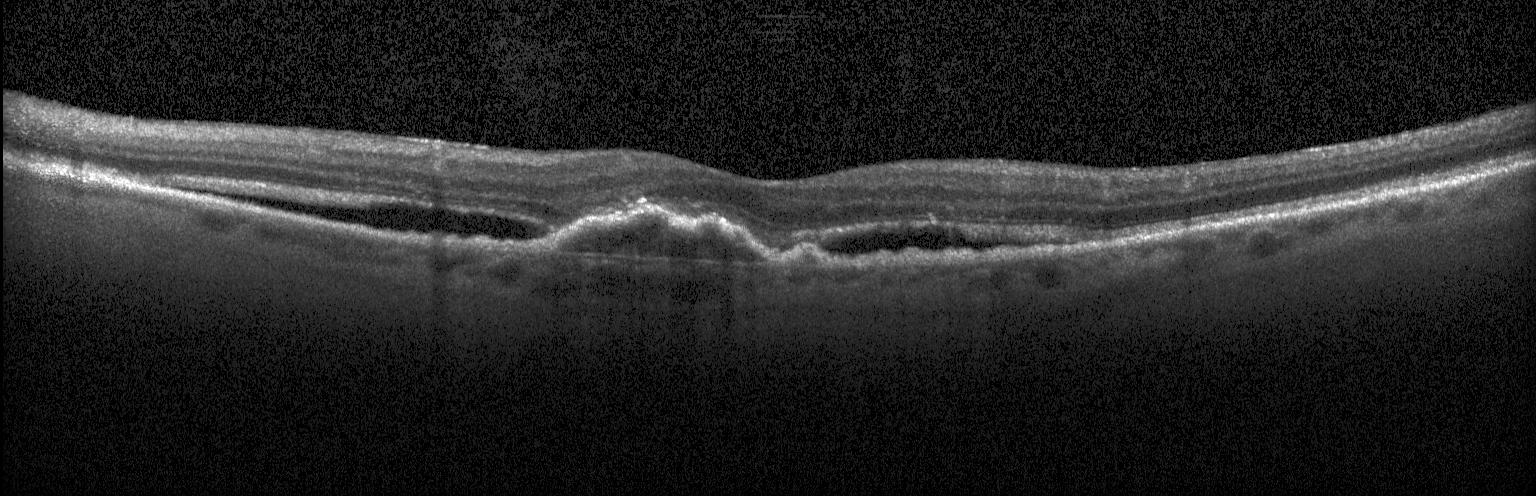

Fovea-centered. Acquired on a Heidelberg Spectralis. Retinal OCT cross-section. Spectral-domain OCT. Diagnosis: a choroidal neovascular membrane.